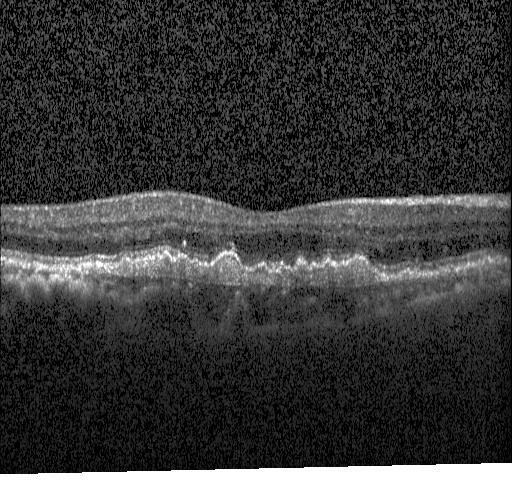
Optical coherence tomography scan · Heidelberg Spectralis OCT system · SD-OCT — The scan shows a choroidal neovascular membrane.